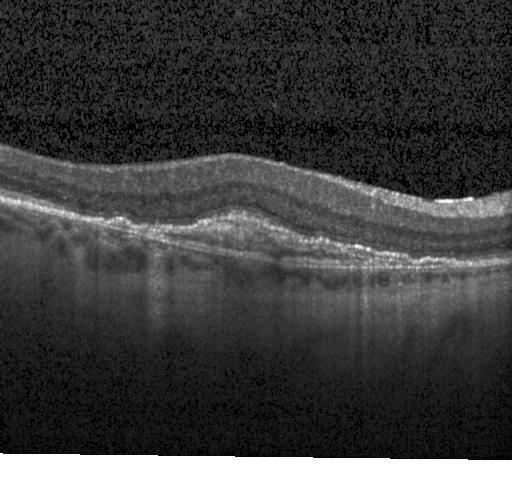 Macular OCT: a choroidal neovascular membrane.